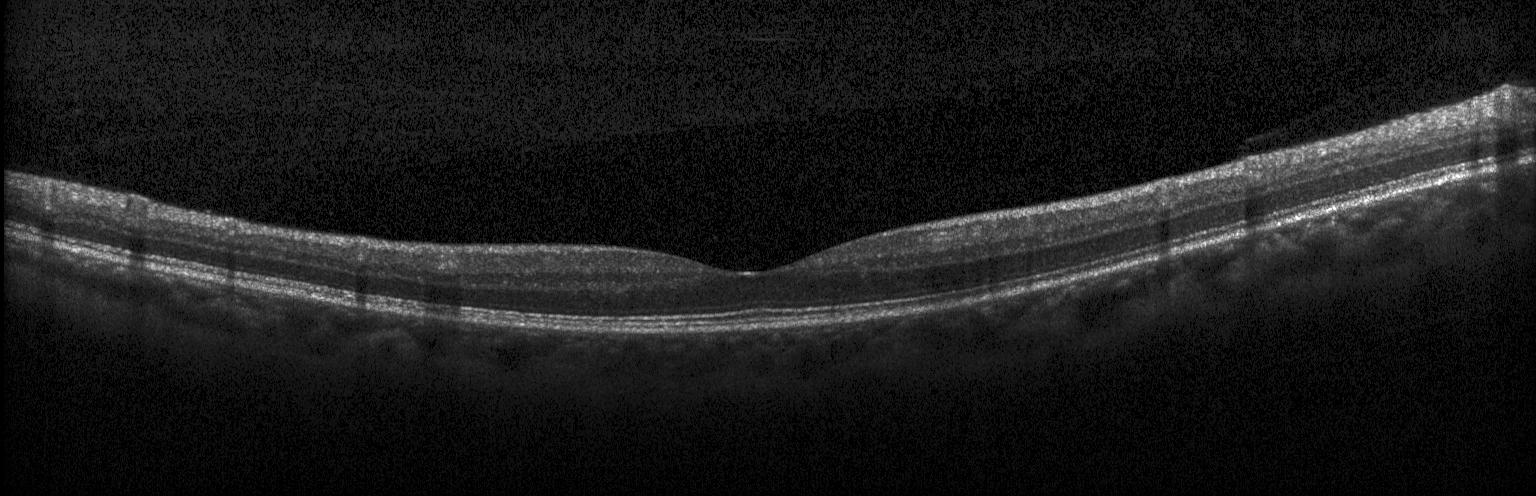
OCT B-scan showing no CNV, no DME, and no drusen.